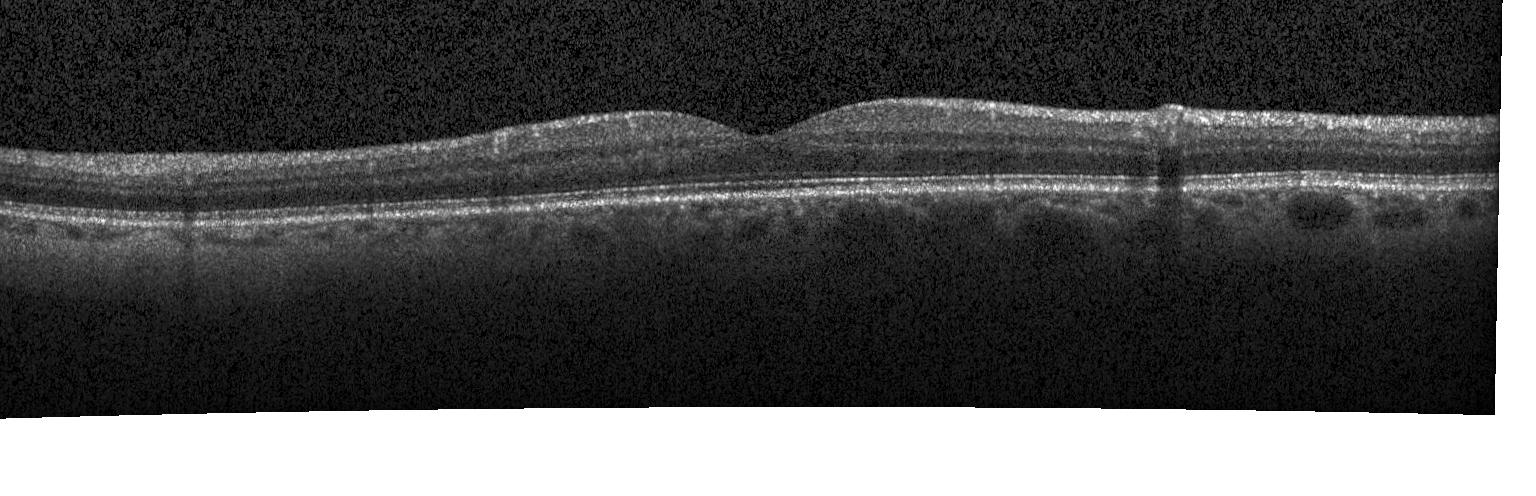

Diagnosis: no CNV, no DME, and no drusen.